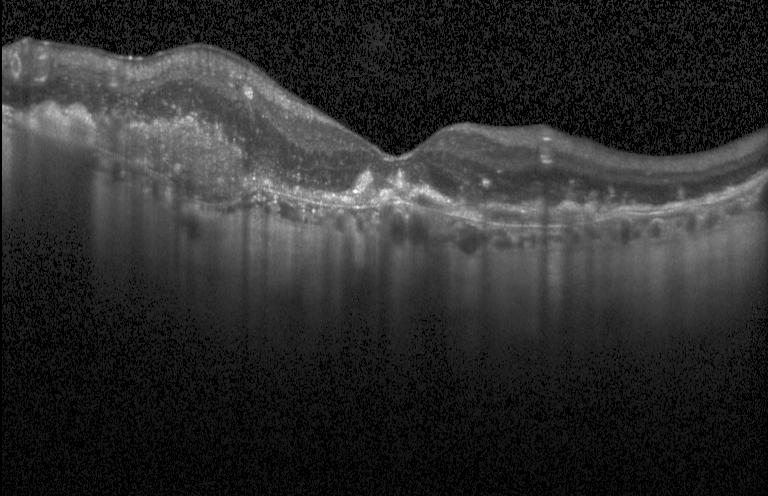

OCT B-scan · Heidelberg Spectralis
Assessment: CNV.